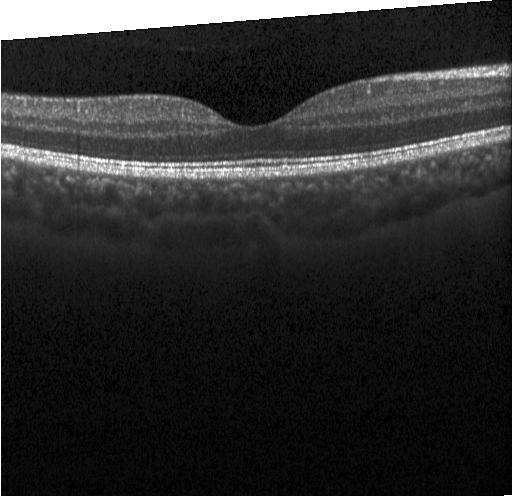
Finding: no CNV, no DME, and no drusen.